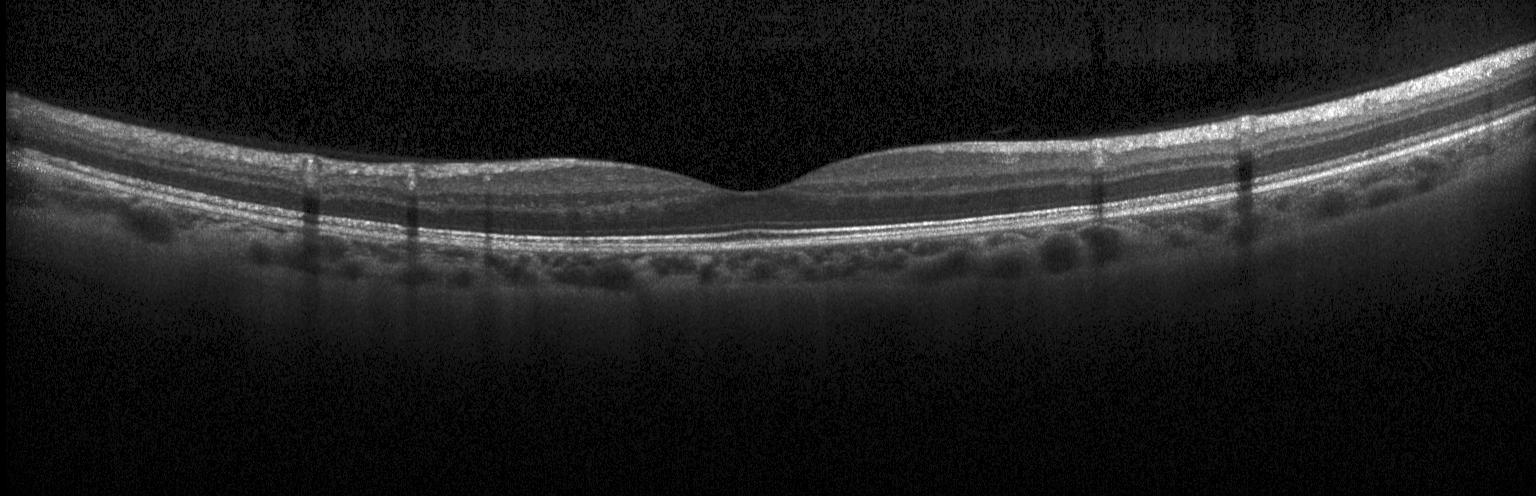

Spectral-domain optical coherence tomography · OCT B-scan · horizontal scan through the fovea.
Assessment: no evidence of choroidal neovascularization, diabetic macular edema, or drusen.